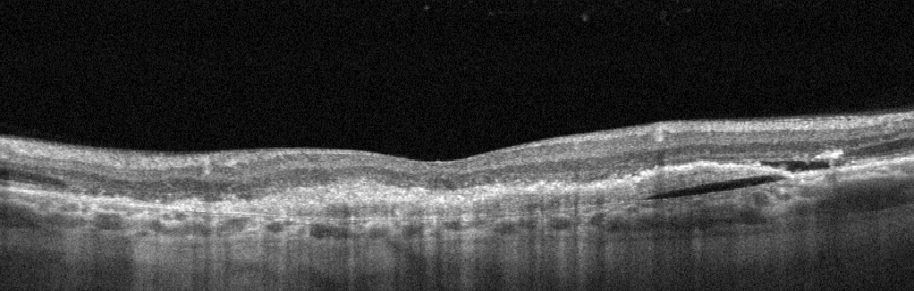

OD; optical coherence tomography scan — The scan shows AMD.